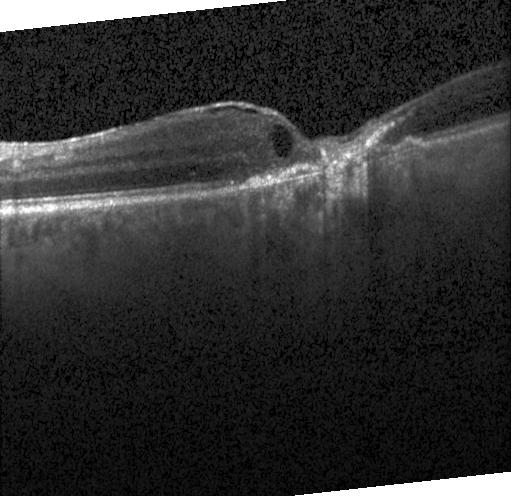

Retinal OCT B-scan. Instrument: Heidelberg Spectralis.
Macular OCT: a choroidal neovascular membrane.